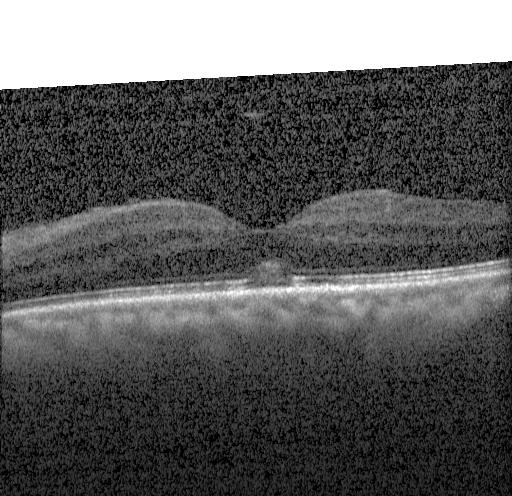

Macular scan · retinal OCT B-scan — This B-scan demonstrates CNV.